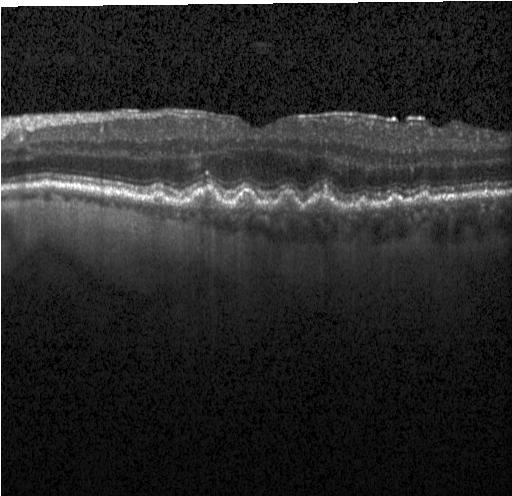

Retinal OCT cross-section, SD-OCT. Dx: sub-RPE drusenoid deposits.